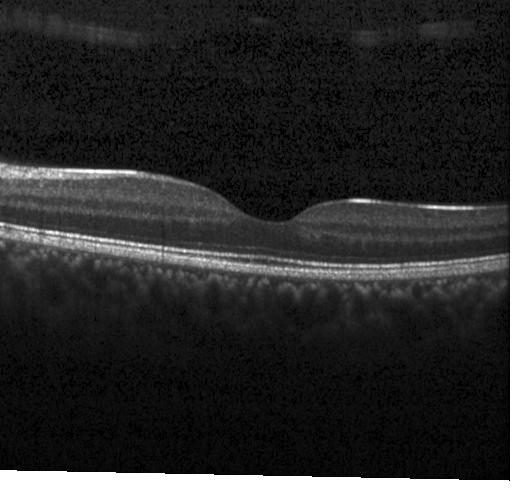
Dx: no choroidal neovascularization, diabetic macular edema, or drusen.